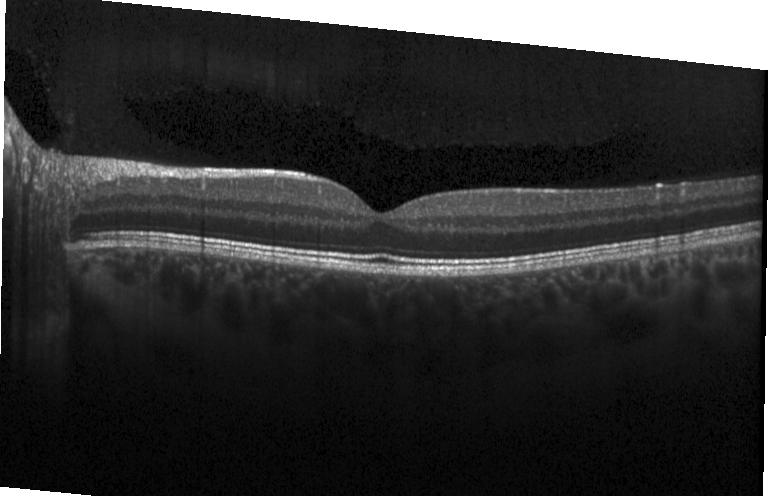 No evidence of choroidal neovascularization, diabetic macular edema, or drusen.